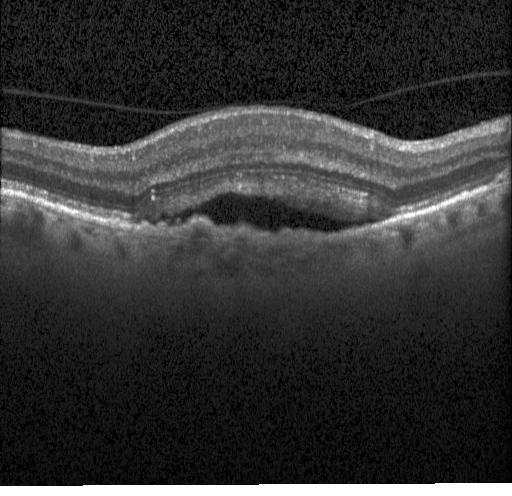 Impression: a choroidal neovascular membrane.